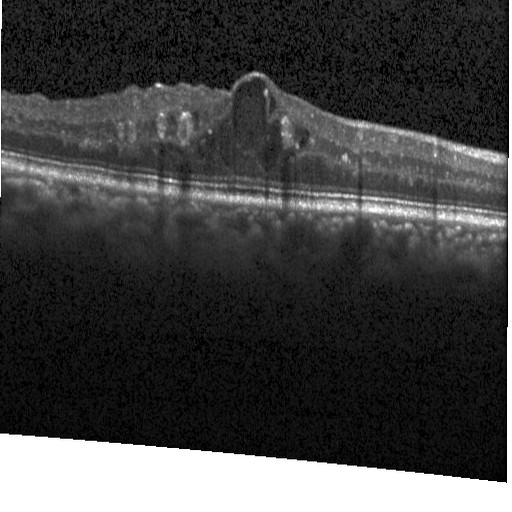 Finding: diabetic macular edema (DME).